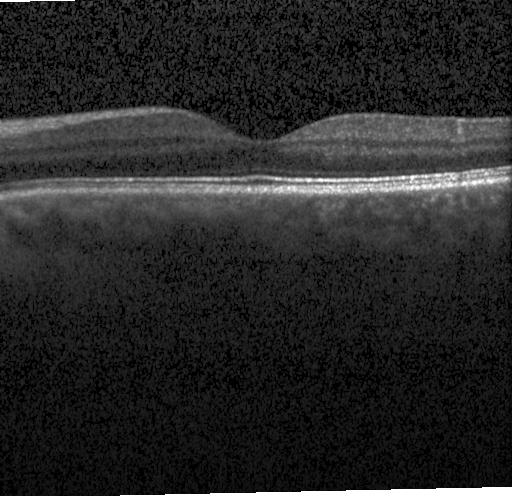
Spectral-domain OCT; through the macula; OCT line scan; acquired on a Heidelberg Spectralis.
Diagnosis: no choroidal neovascularization, diabetic macular edema, or drusen.